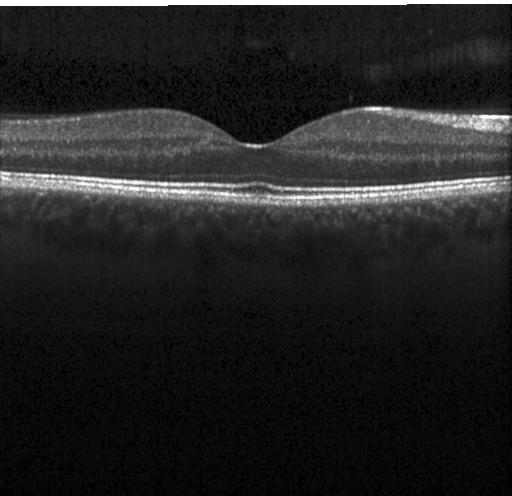 Fovea-centered · optical coherence tomography B-scan.
Dx: no choroidal neovascularization, diabetic macular edema, or drusen.